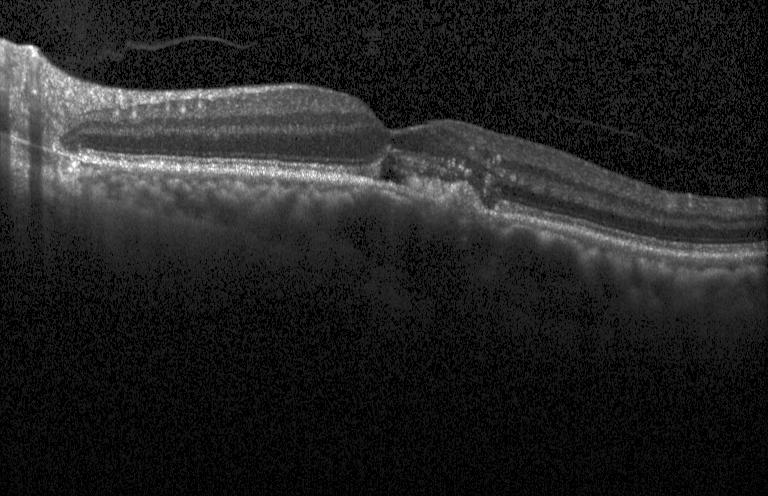 SD-OCT, optical coherence tomography scan, through the macula.
Dx: a choroidal neovascular membrane.